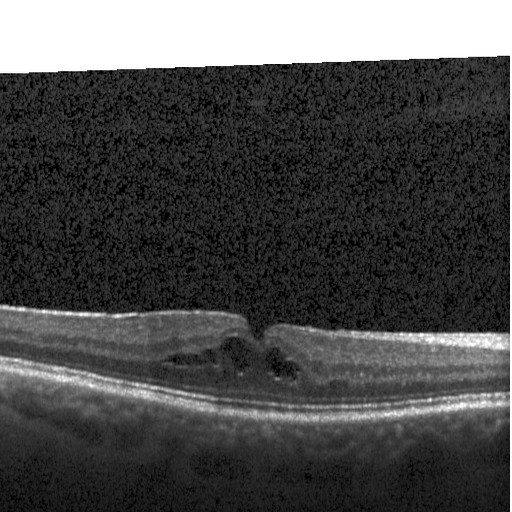

SD-OCT; macular scan; Heidelberg Spectralis OCT system; retinal OCT cross-section
Diagnosis: diabetic macular edema.